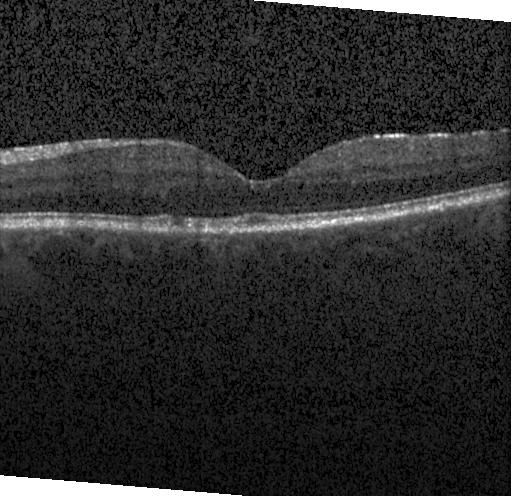
Instrument: Heidelberg Spectralis; retinal OCT cross-section; fovea-centered. Finding: no evidence of choroidal neovascularization, diabetic macular edema, or drusen.